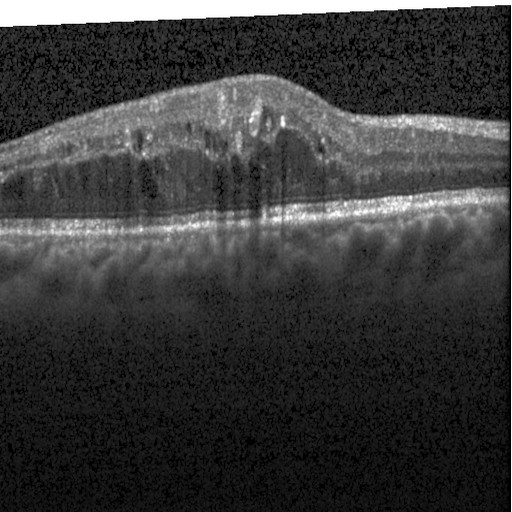

OCT scan showing diabetic macular edema.